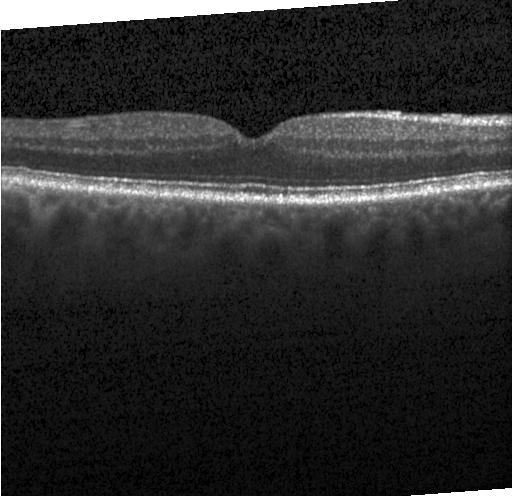

Fovea-centered · retinal OCT B-scan
This B-scan demonstrates no choroidal neovascularization, diabetic macular edema, or drusen.